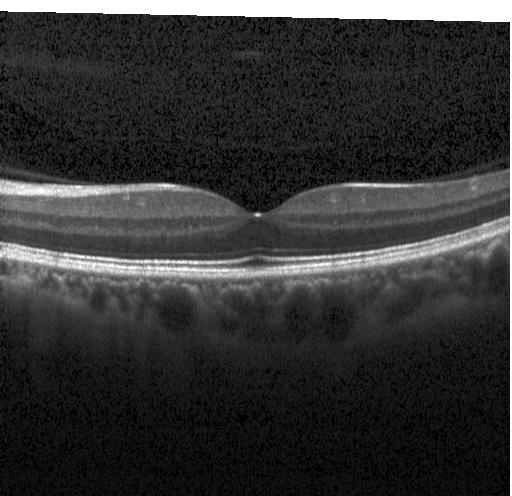 This B-scan demonstrates neither CNV, DME, nor drusen.